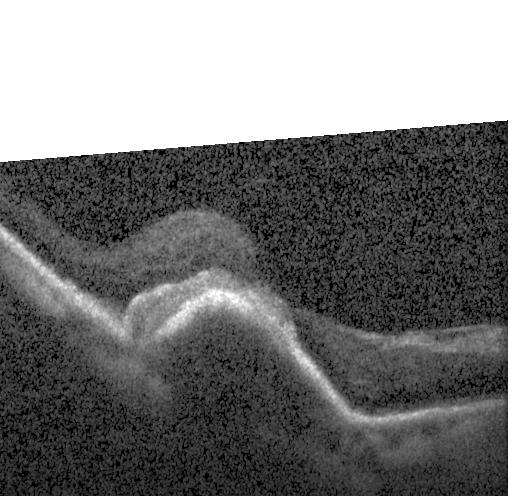
Optical coherence tomography B-scan
Assessment: a choroidal neovascular membrane.